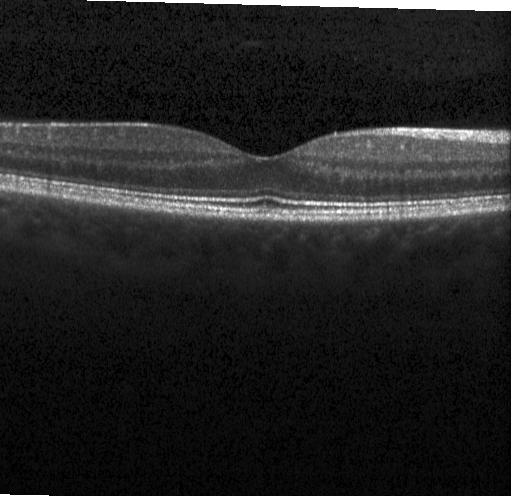

Optical coherence tomography B-scan
Macular OCT: neither CNV, DME, nor drusen.